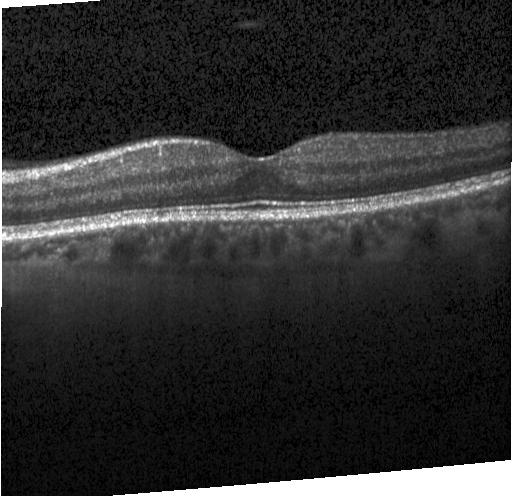 OCT line scan, SD-OCT, horizontal scan through the fovea, Heidelberg Spectralis OCT system
The scan shows no choroidal neovascularization, diabetic macular edema, or drusen.